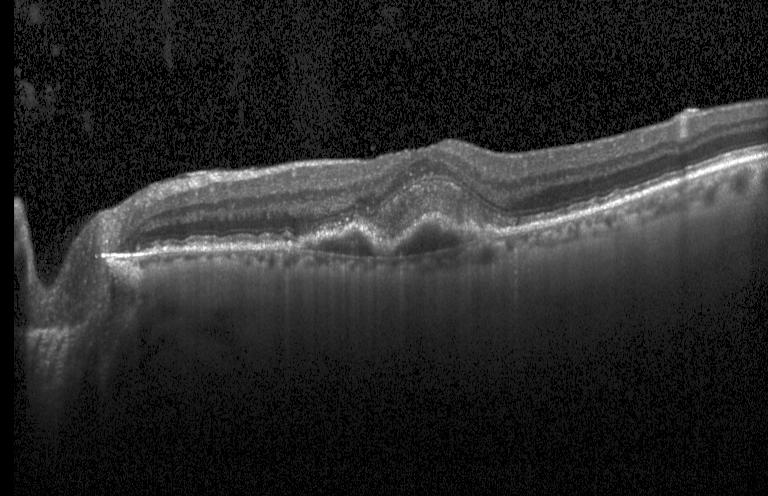

Macular scan, spectral-domain OCT, retinal OCT B-scan, Heidelberg Spectralis OCT system.
Assessment: a choroidal neovascular membrane.